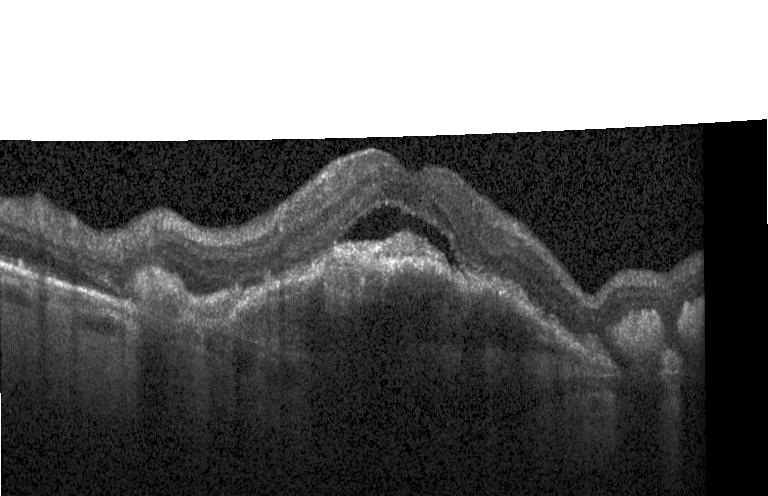 Optical coherence tomography scan.
Assessment: CNV.